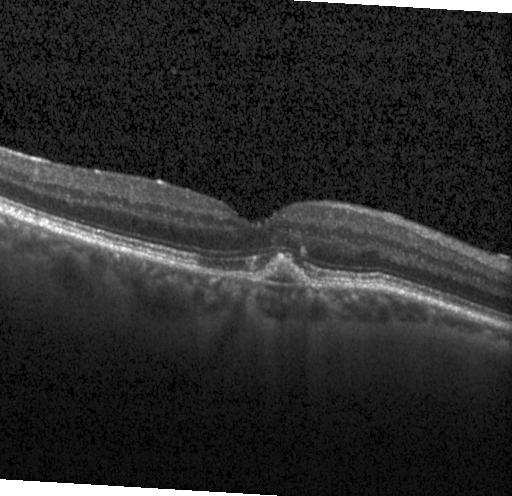
Optical coherence tomography B-scan; Heidelberg Spectralis; spectral-domain optical coherence tomography; through the macula.
Diagnosis: choroidal neovascularization (CNV).